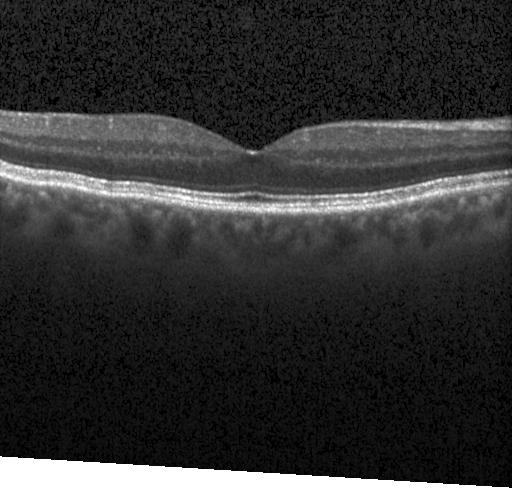 OCT scan showing no evidence of CNV, DME, or drusen.